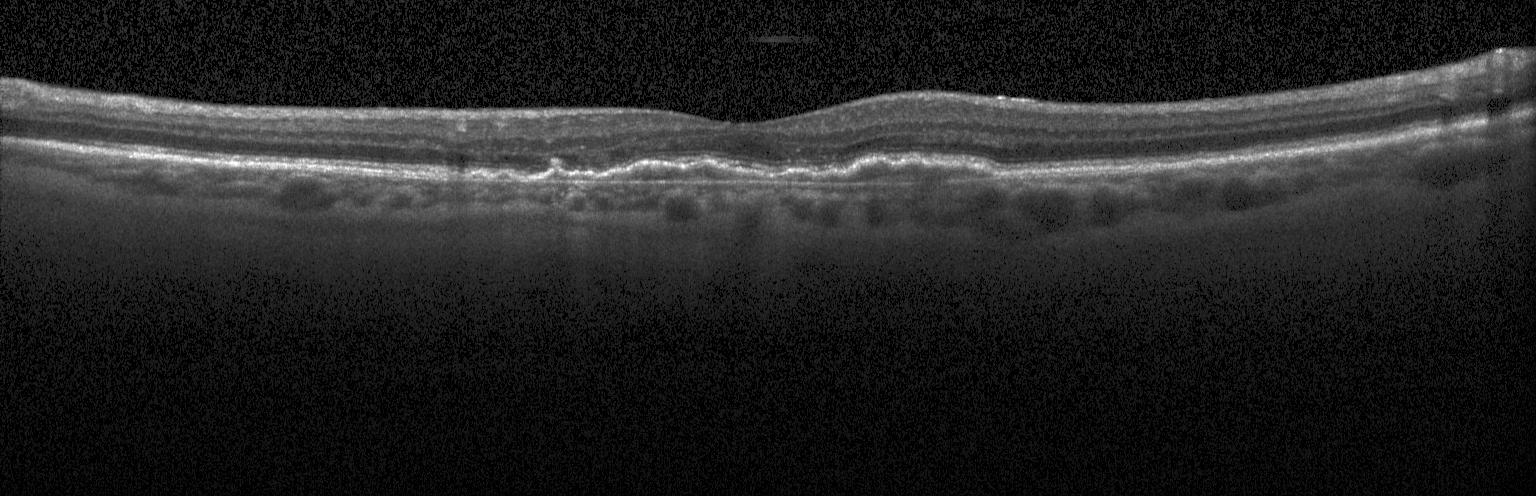

Through the macula; instrument: Heidelberg Spectralis; SD-OCT; optical coherence tomography B-scan.
Assessment: CNV.